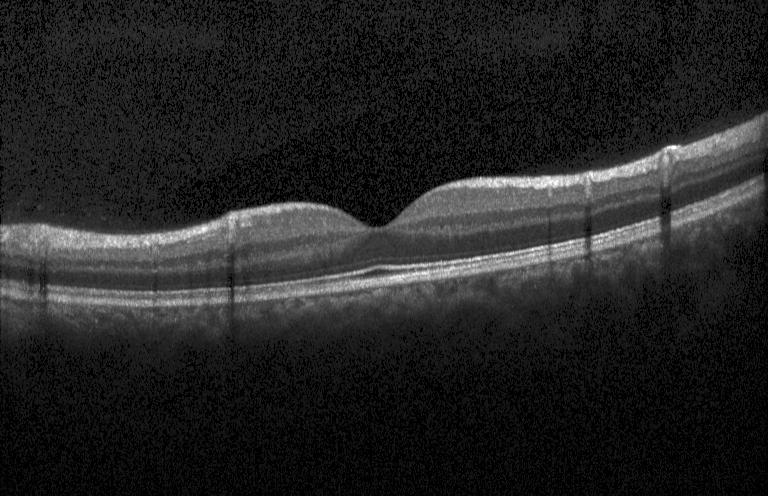 OCT line scan.
The scan shows no choroidal neovascularization, no diabetic macular edema, and no drusen.